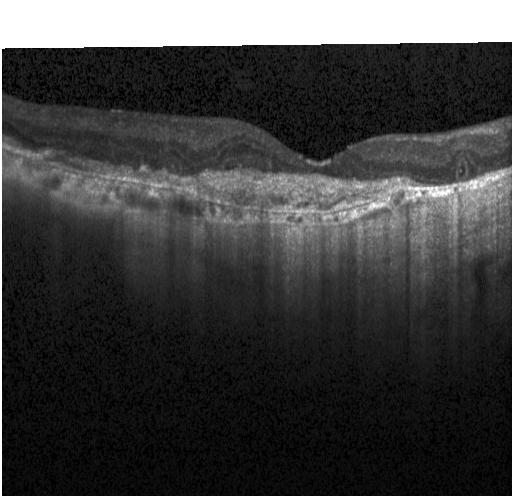

Optical coherence tomography B-scan.
Finding: choroidal neovascularization.